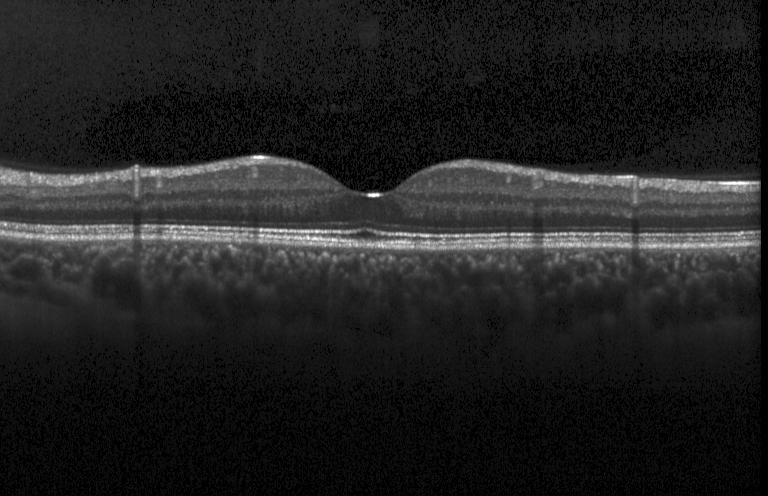
Horizontal scan through the fovea, Heidelberg Spectralis, SD-OCT, OCT B-scan. Diagnosis: no choroidal neovascularization, no diabetic macular edema, and no drusen.